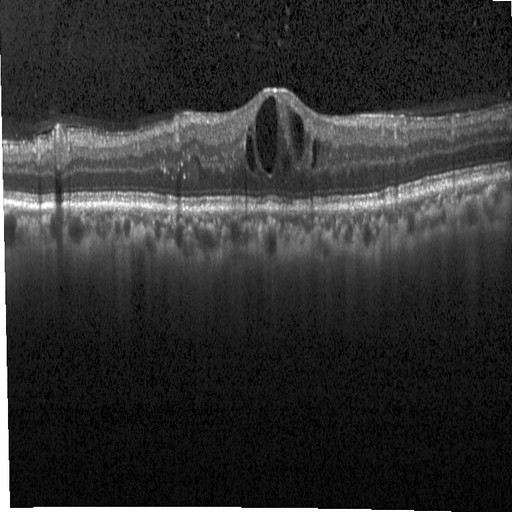
OCT line scan; Heidelberg Spectralis — Assessment: diabetic macular edema (DME).